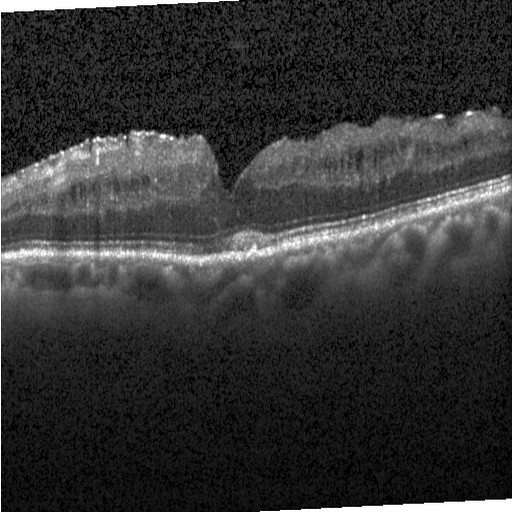 OCT scan showing diabetic macular edema.